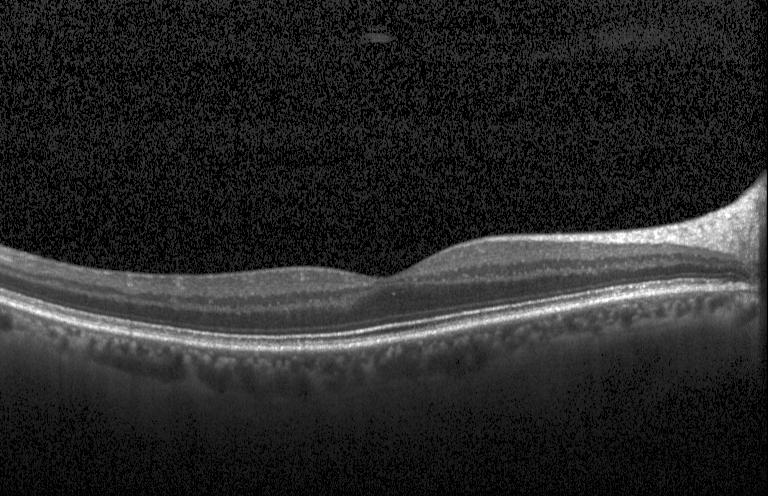

Optical coherence tomography B-scan, through the macula, spectral-domain optical coherence tomography.
OCT finding: no evidence of choroidal neovascularization, diabetic macular edema, or drusen.